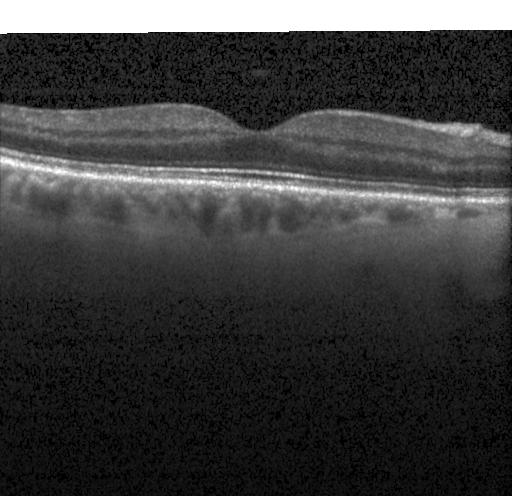 Acquired on a Heidelberg Spectralis. Macular scan. SD-OCT. OCT line scan. Impression: no choroidal neovascularization, no diabetic macular edema, and no drusen.